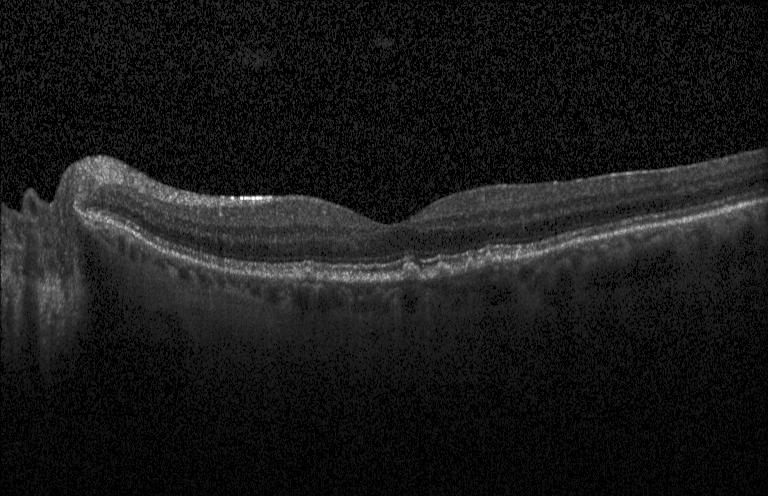

Retinal OCT cross-section showing drusen.